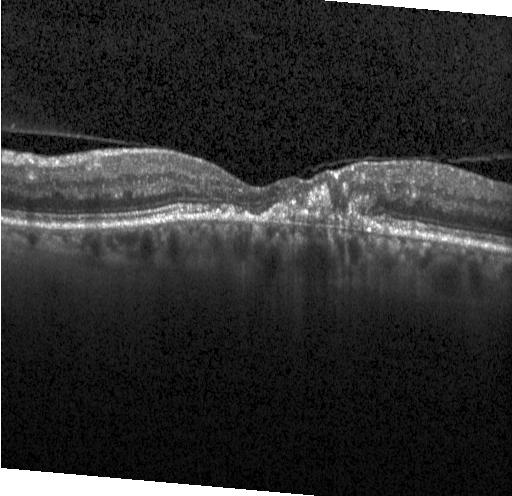 Heidelberg Spectralis. Through the macula. Spectral-domain OCT. OCT B-scan
Diagnosis: a choroidal neovascular membrane.